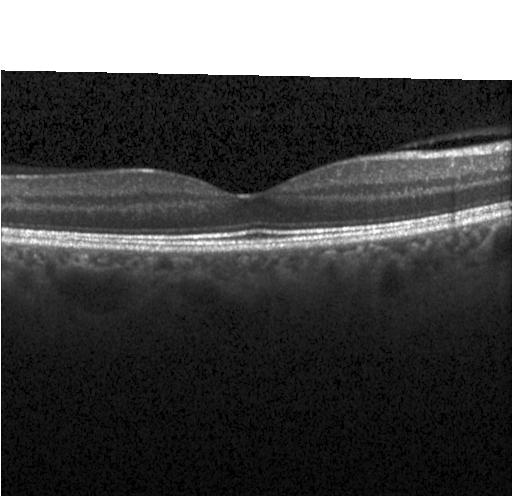
Optical coherence tomography scan — Diagnosis: no evidence of choroidal neovascularization, diabetic macular edema, or drusen.